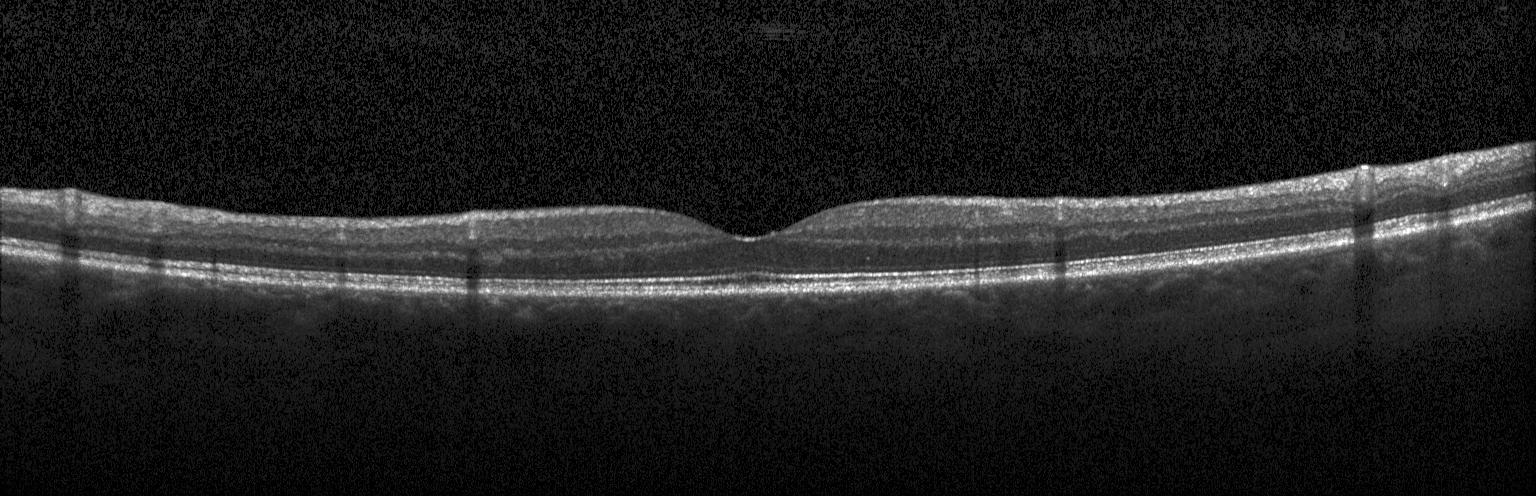
OCT B-scan showing no evidence of choroidal neovascularization, diabetic macular edema, or drusen.